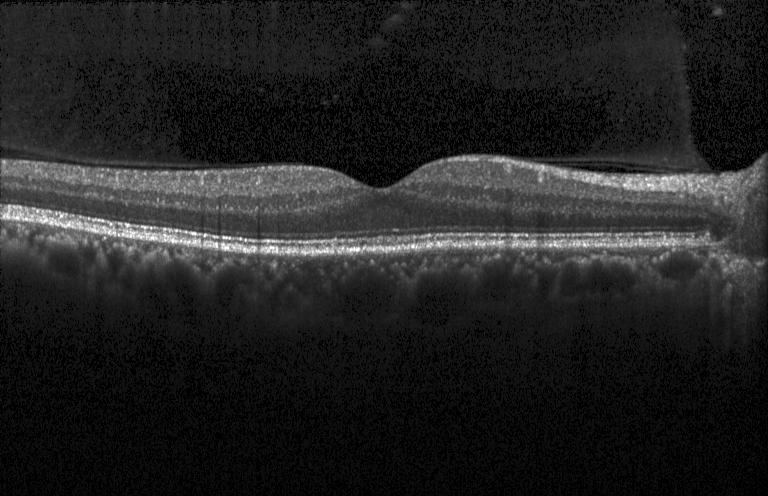
Macular scan, acquired on a Heidelberg Spectralis, retinal OCT B-scan, SD-OCT — The scan shows no choroidal neovascularization, diabetic macular edema, or drusen.